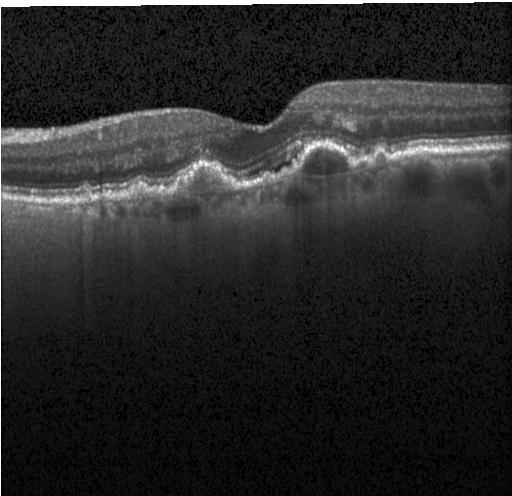

Finding: a choroidal neovascular membrane.